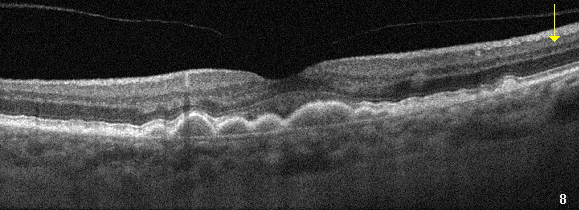 Retinal OCT B-scan
Diagnosis: AMD.